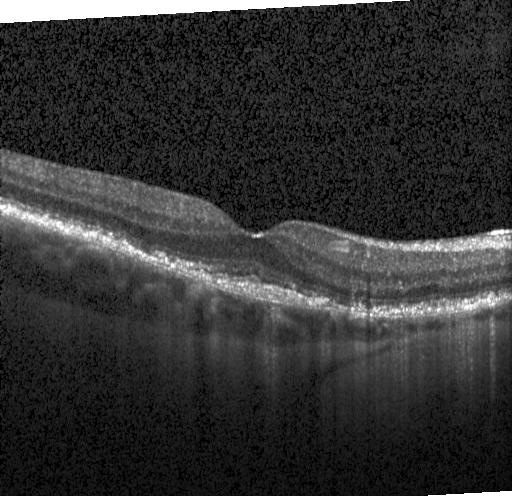
Centered on the fovea; SD-OCT; OCT B-scan; Heidelberg Spectralis OCT system.
CNV.